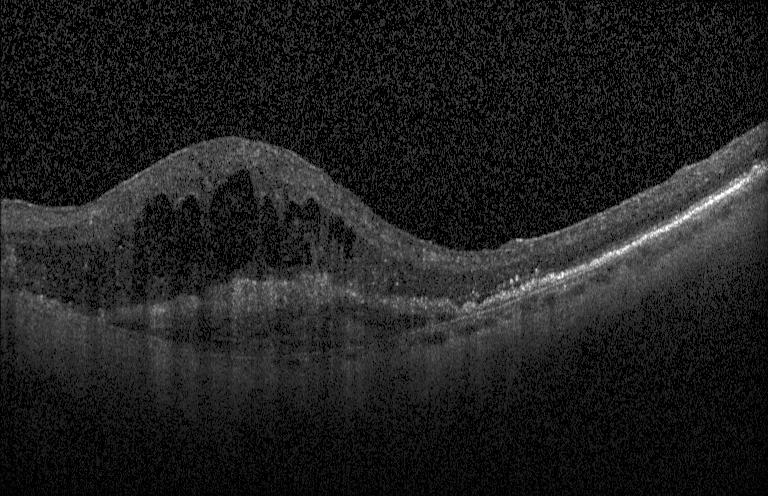 Dx: a choroidal neovascular membrane.